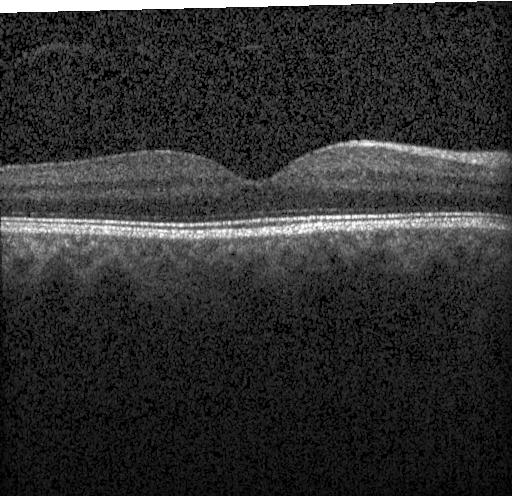 Acquired on a Heidelberg Spectralis, SD-OCT, horizontal scan through the fovea, retinal OCT B-scan — Finding: no choroidal neovascularization, no diabetic macular edema, and no drusen.